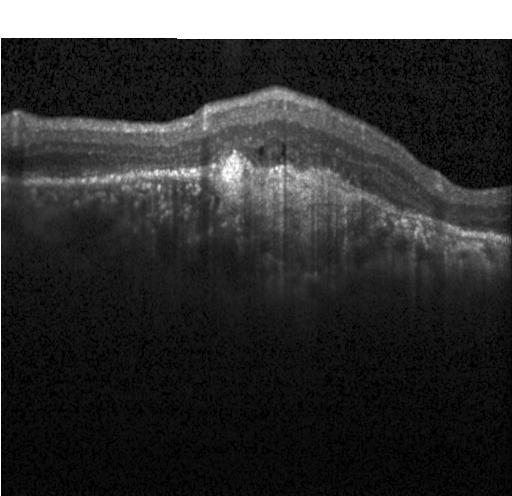
Spectral-domain optical coherence tomography · retinal OCT cross-section · horizontal scan through the fovea
Diagnosis: choroidal neovascularization (CNV).